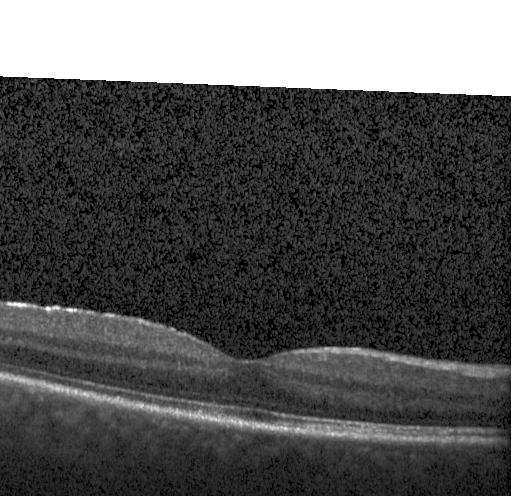 This B-scan demonstrates no choroidal neovascularization, no diabetic macular edema, and no drusen.